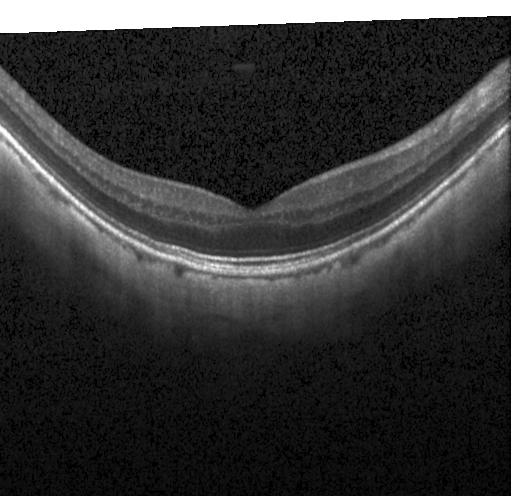

Instrument: Heidelberg Spectralis · through the macula · spectral-domain optical coherence tomography · optical coherence tomography scan
OCT finding: no choroidal neovascularization, diabetic macular edema, or drusen.